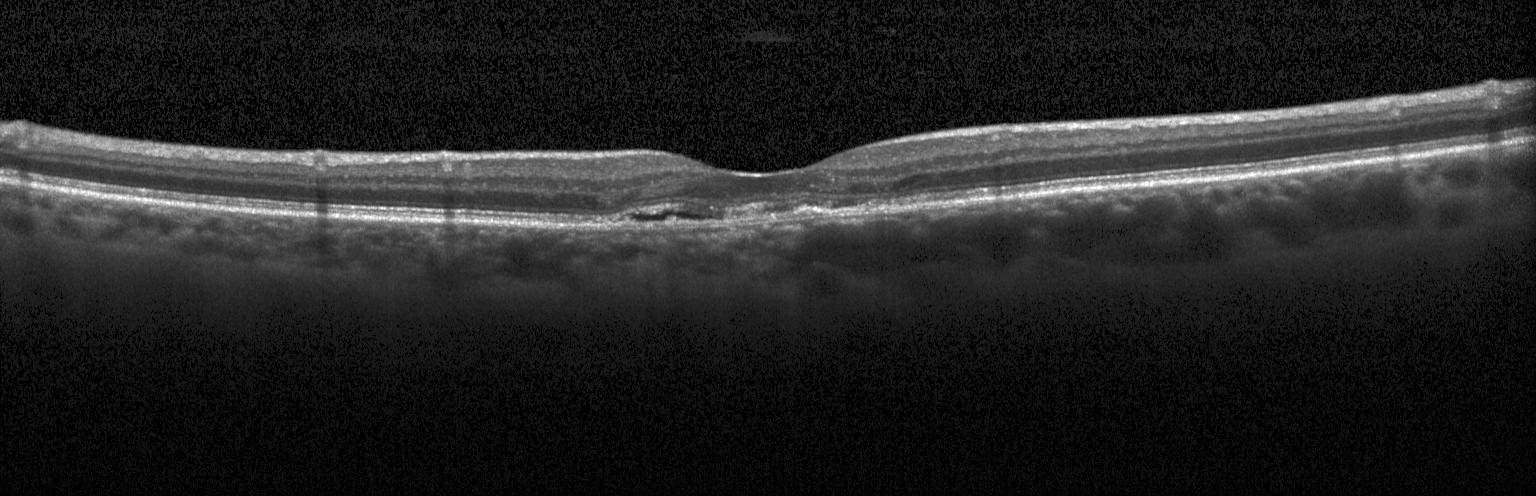
SD-OCT · retinal OCT B-scan — This B-scan demonstrates a choroidal neovascular membrane.